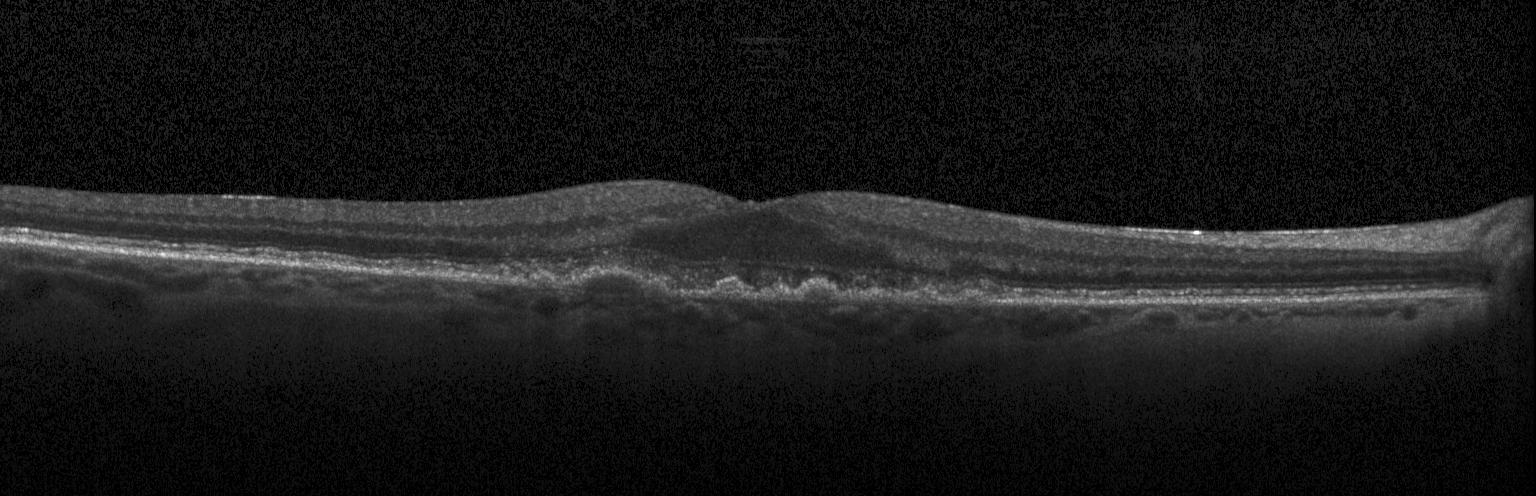
Optical coherence tomography scan — Macular OCT: sub-RPE drusenoid deposits.